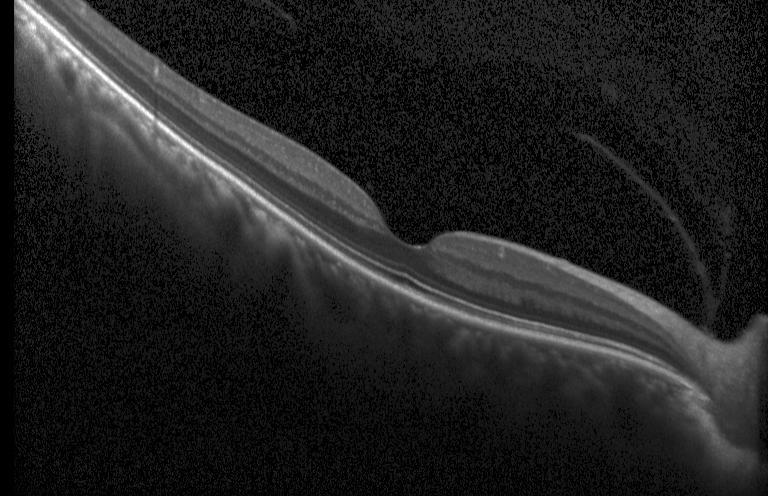 OCT finding: neither choroidal neovascularization, diabetic macular edema, nor drusen.